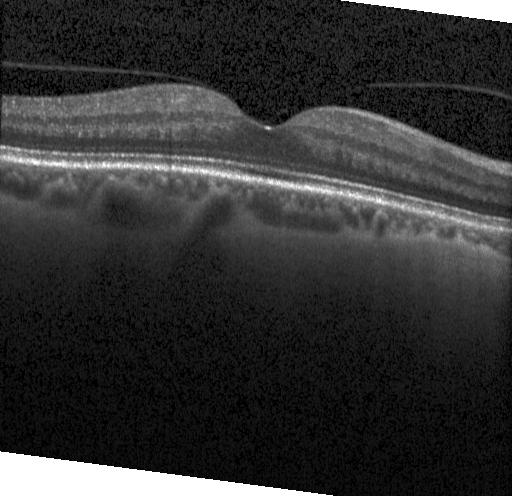
Heidelberg Spectralis · OCT B-scan · spectral-domain optical coherence tomography — This B-scan demonstrates no evidence of choroidal neovascularization, diabetic macular edema, or drusen.